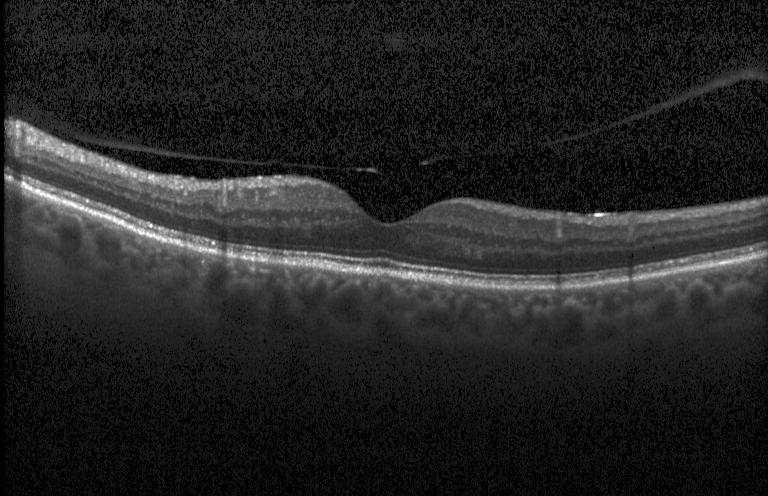
Retinal OCT B-scan
Diagnosis: neither choroidal neovascularization, diabetic macular edema, nor drusen.